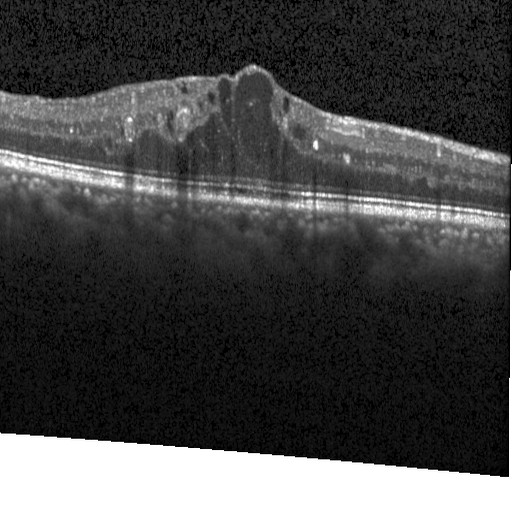

OCT line scan; centered on the fovea; Heidelberg Spectralis. OCT finding: diabetic macular edema (DME).